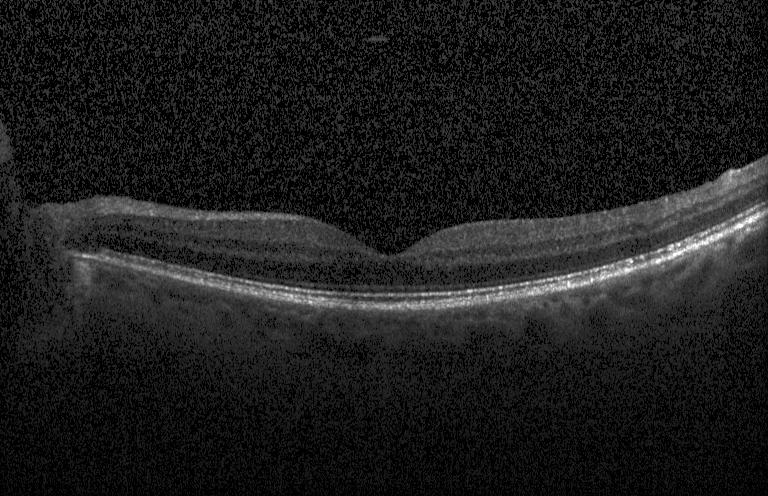
Optical coherence tomography scan — Finding: neither choroidal neovascularization, diabetic macular edema, nor drusen.